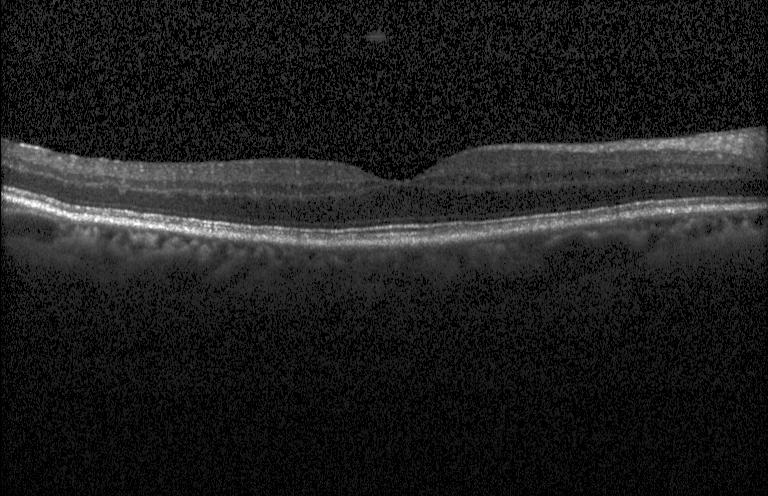
Retinal OCT cross-section showing neither CNV, DME, nor drusen.